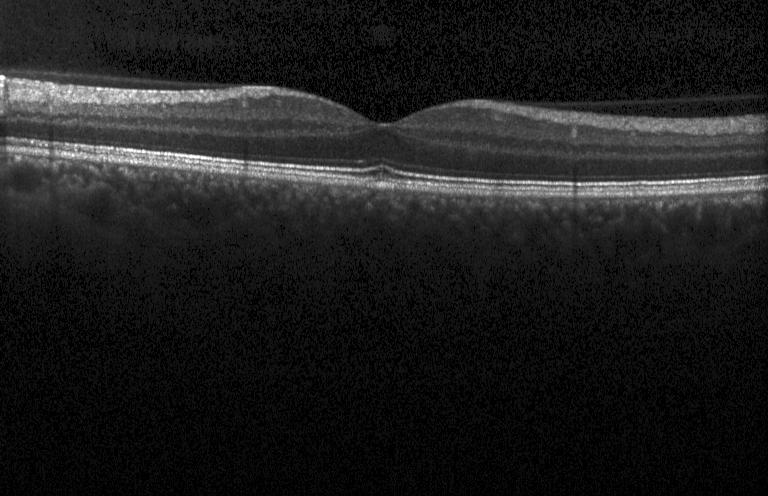 Impression: neither choroidal neovascularization, diabetic macular edema, nor drusen.